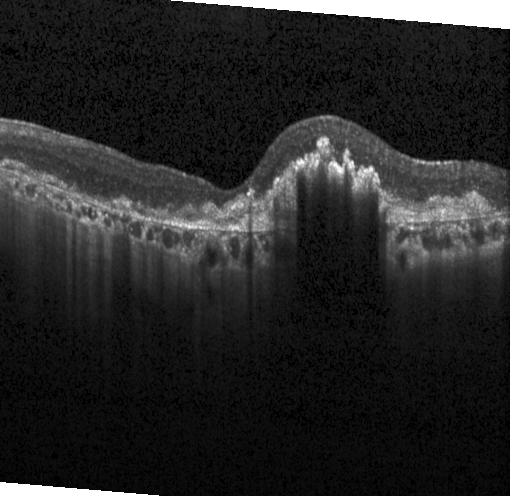 Fovea-centered. Optical coherence tomography B-scan. Diagnosis: choroidal neovascularization.